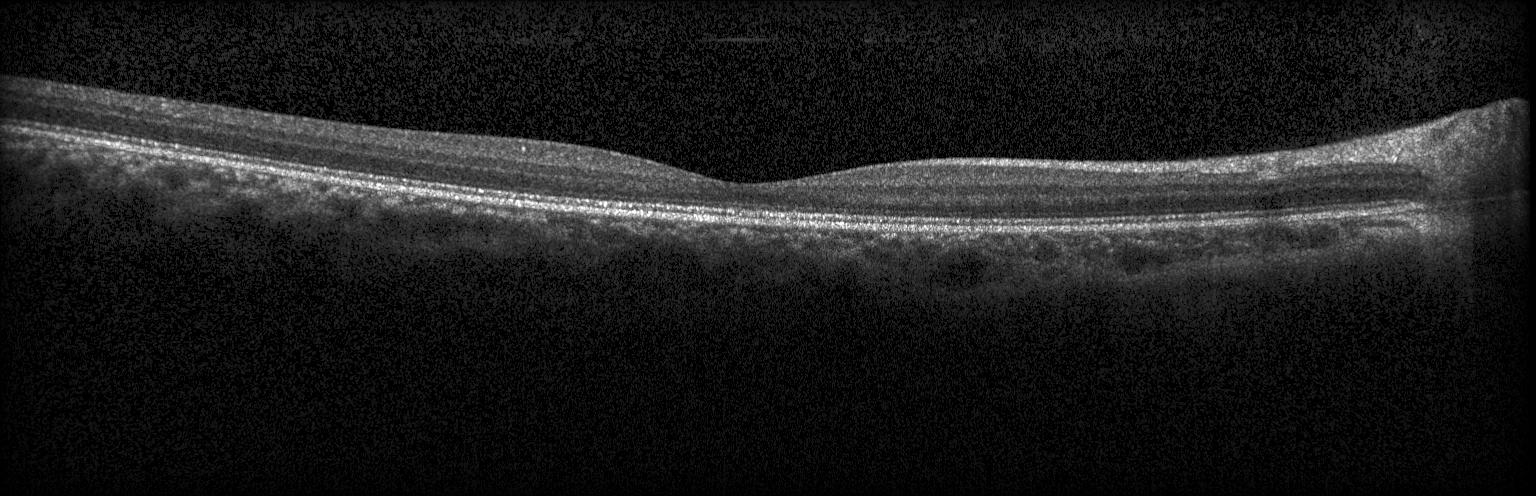
Optical coherence tomography scan · macular scan · spectral-domain optical coherence tomography.
Diagnosis: no evidence of choroidal neovascularization, diabetic macular edema, or drusen.